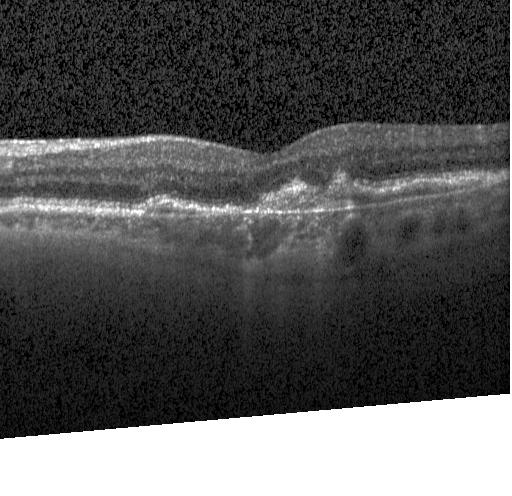

Impression: choroidal neovascularization (CNV).